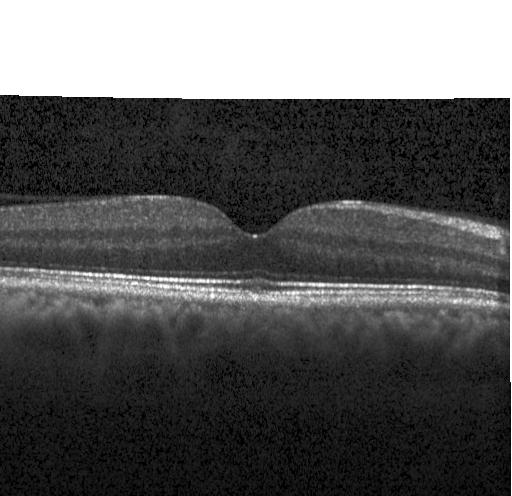
SD-OCT, acquired on a Heidelberg Spectralis, retinal OCT cross-section, centered on the fovea — Finding: no choroidal neovascularization, no diabetic macular edema, and no drusen.